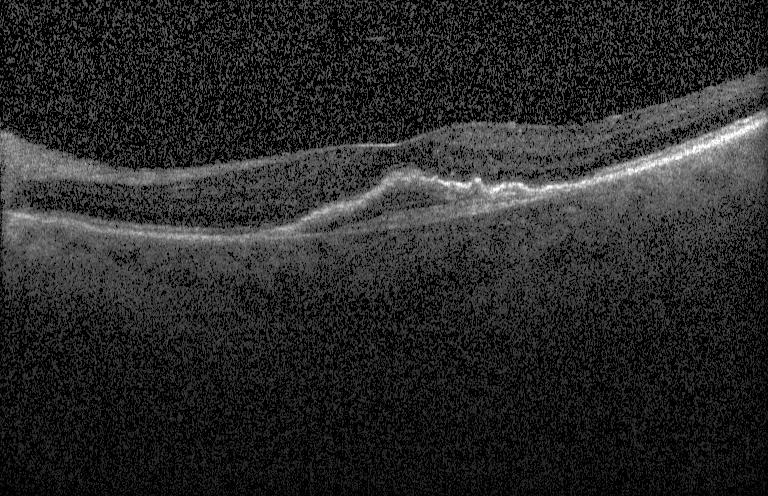
Impression: a choroidal neovascular membrane.